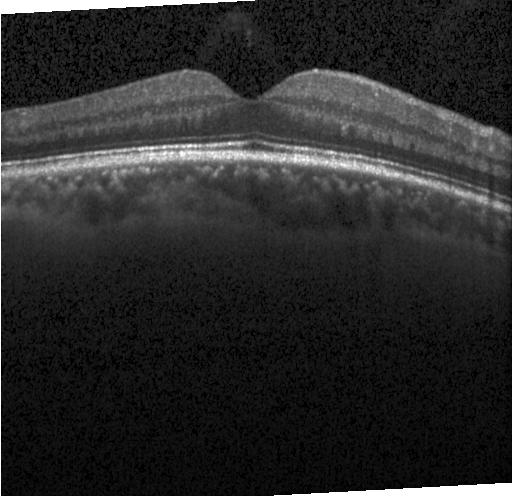

Fovea-centered, OCT B-scan
This B-scan demonstrates no choroidal neovascularization, no diabetic macular edema, and no drusen.